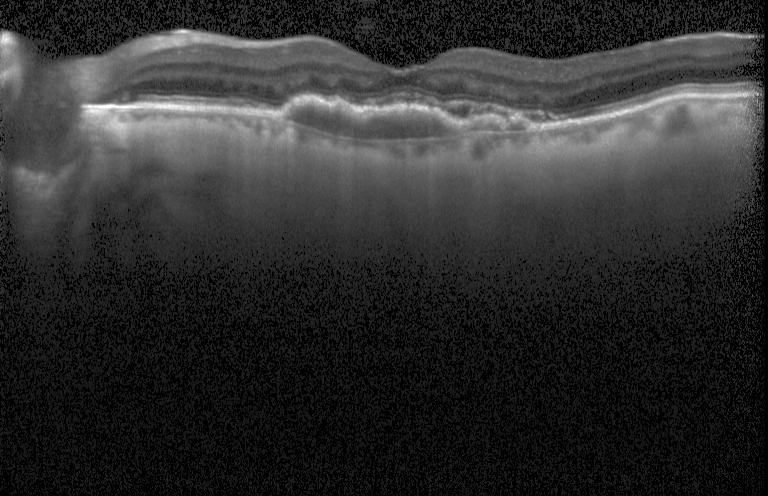
Spectral-domain optical coherence tomography, Heidelberg Spectralis, OCT B-scan, centered on the fovea — Diagnosis: a choroidal neovascular membrane.